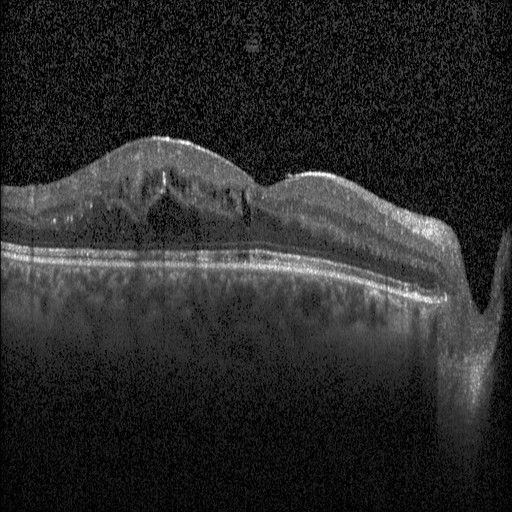
OCT finding: diabetic macular edema.